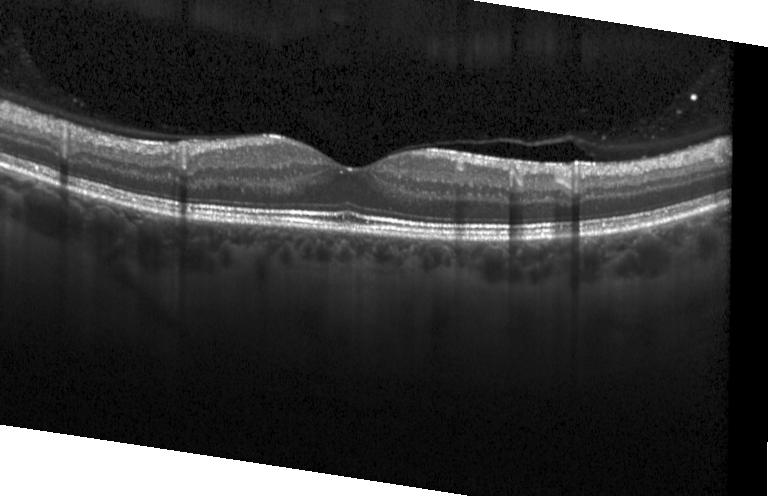 Macular OCT: no evidence of choroidal neovascularization, diabetic macular edema, or drusen.